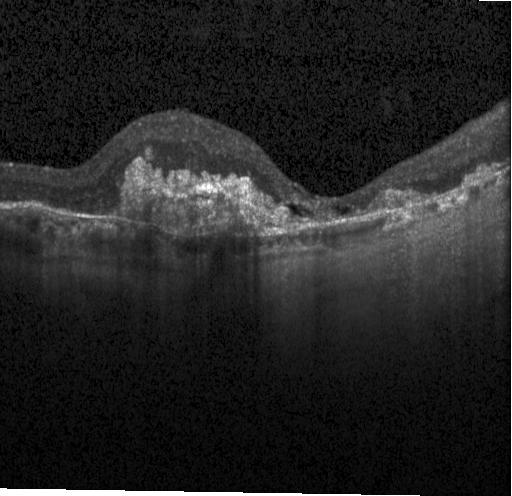 Optical coherence tomography scan — This B-scan demonstrates a choroidal neovascular membrane.